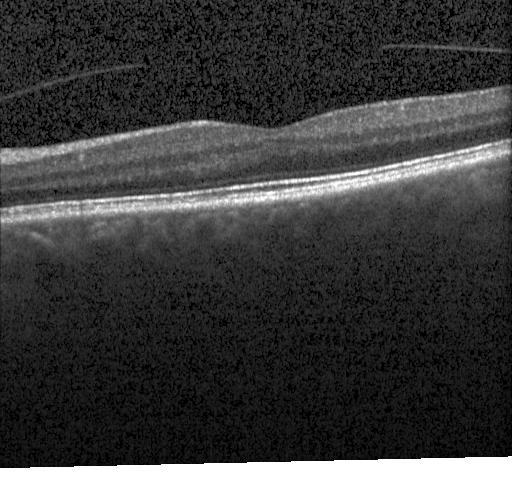

Retinal OCT cross-section — This B-scan demonstrates no choroidal neovascularization, diabetic macular edema, or drusen.